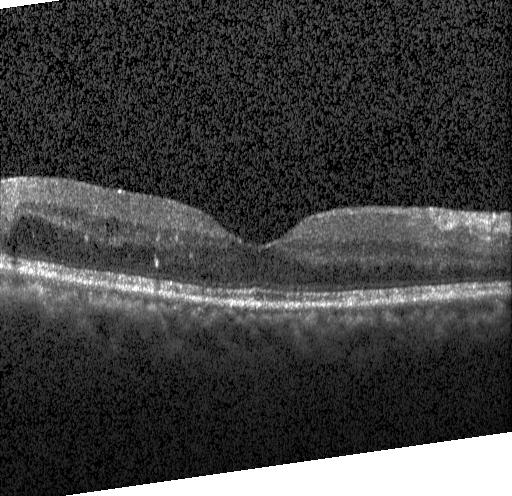 Optical coherence tomography B-scan, through the macula, Heidelberg Spectralis OCT system — Finding: diabetic macular edema (DME).